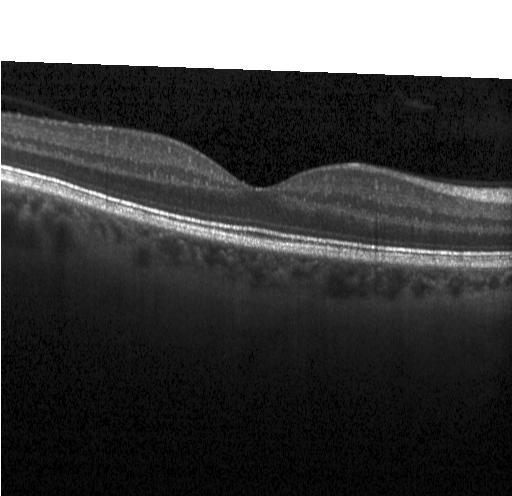 Spectral-domain OCT B-scan: no choroidal neovascularization, diabetic macular edema, or drusen.